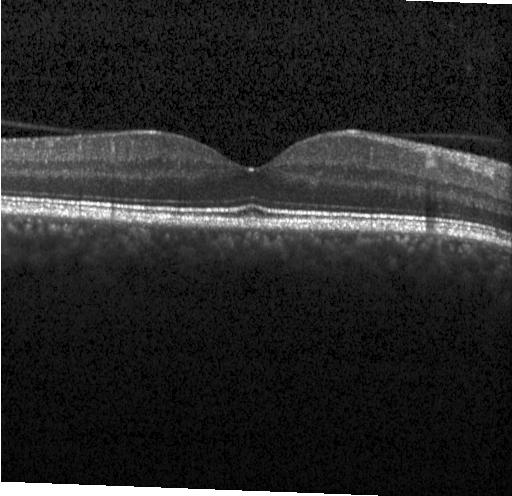
Retinal OCT B-scan. Dx: no choroidal neovascularization, diabetic macular edema, or drusen.